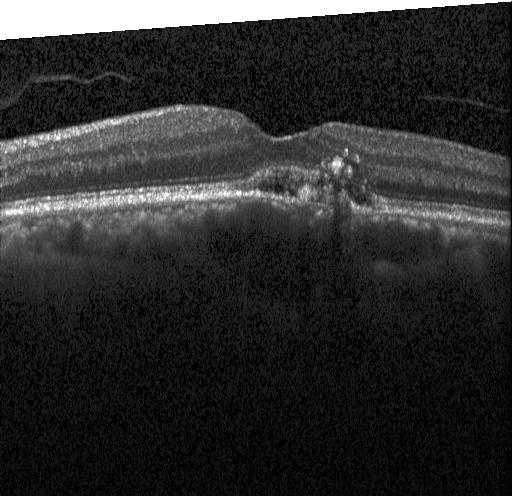 Macular OCT demonstrating choroidal neovascularization.